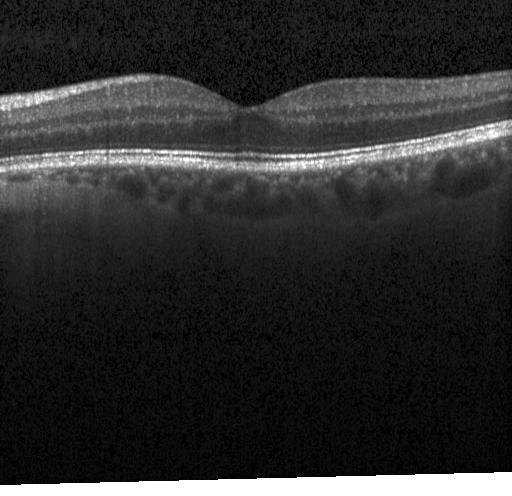

Finding: no CNV, DME, or drusen.